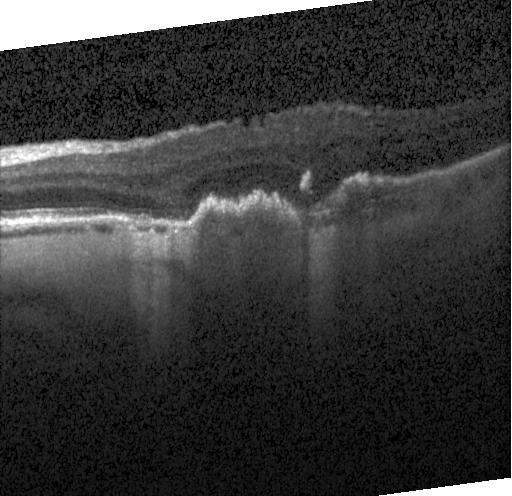

Impression: a choroidal neovascular membrane.